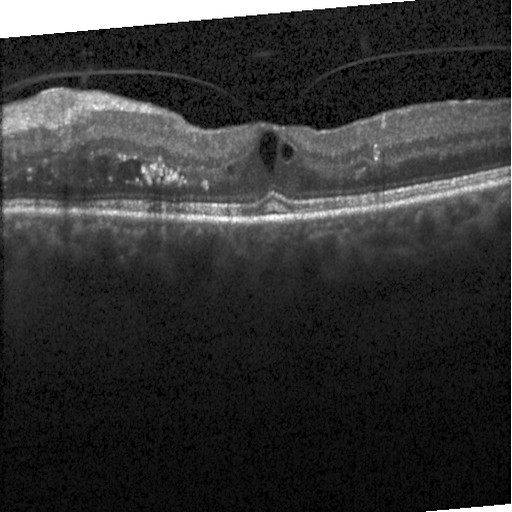
Heidelberg Spectralis OCT system, retinal OCT cross-section. Diagnosis: diabetic macular edema.